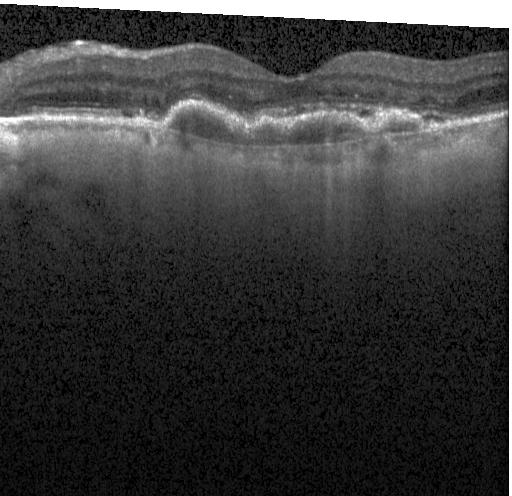
Retinal OCT B-scan. SD-OCT
Dx: a choroidal neovascular membrane.